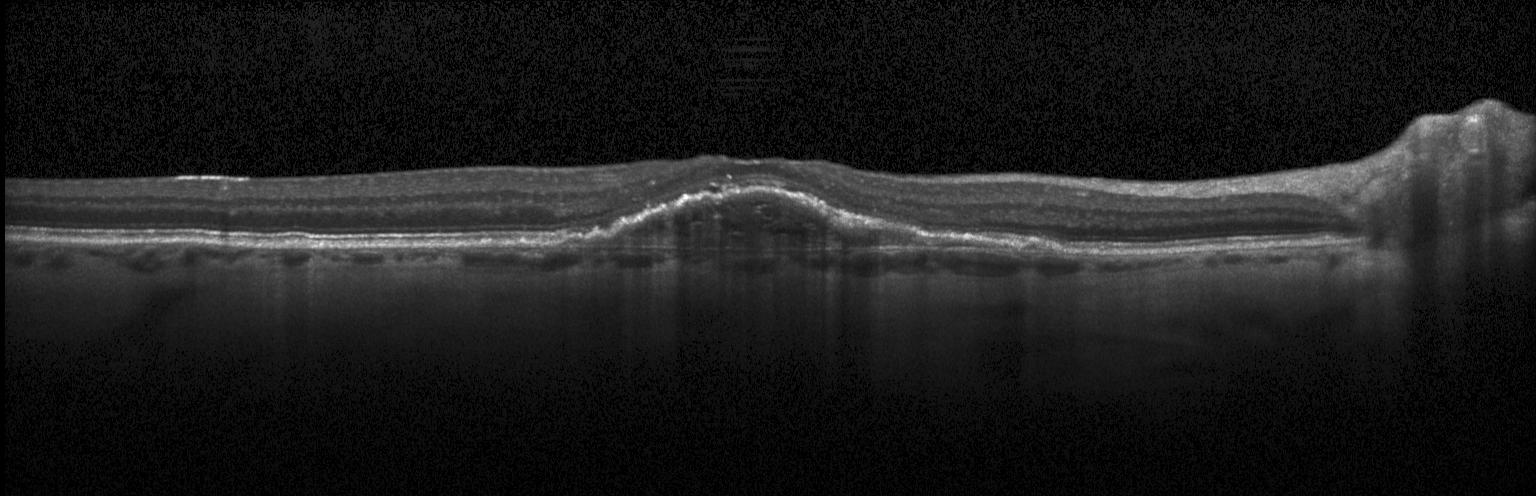

Dx: a choroidal neovascular membrane.